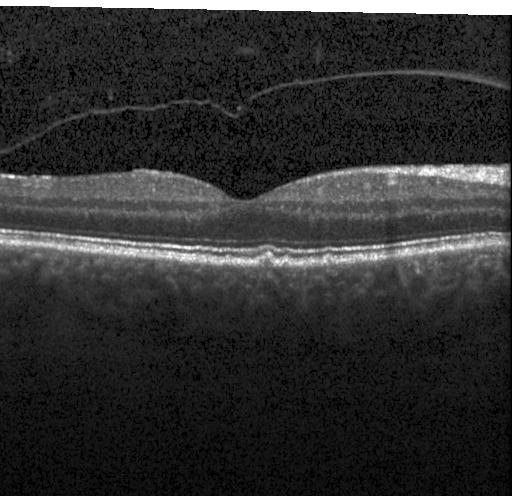

This B-scan demonstrates multiple drusen.